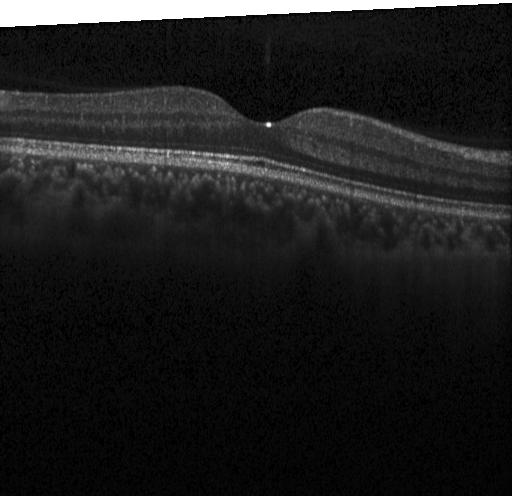

OCT B-scan. Spectral-domain OCT. Fovea-centered
Finding: no choroidal neovascularization, no diabetic macular edema, and no drusen.